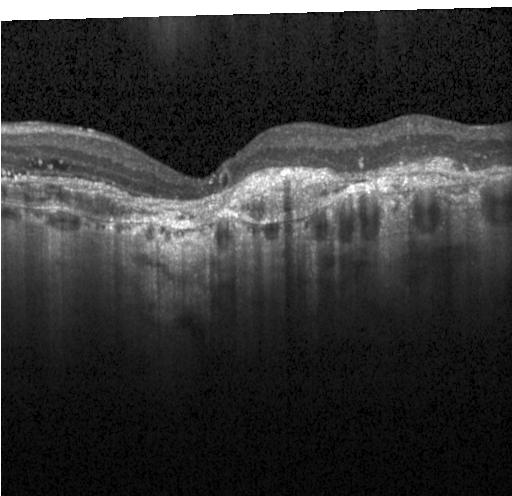
Retinal OCT cross-section, Heidelberg Spectralis, spectral-domain optical coherence tomography.
This B-scan demonstrates a choroidal neovascular membrane.